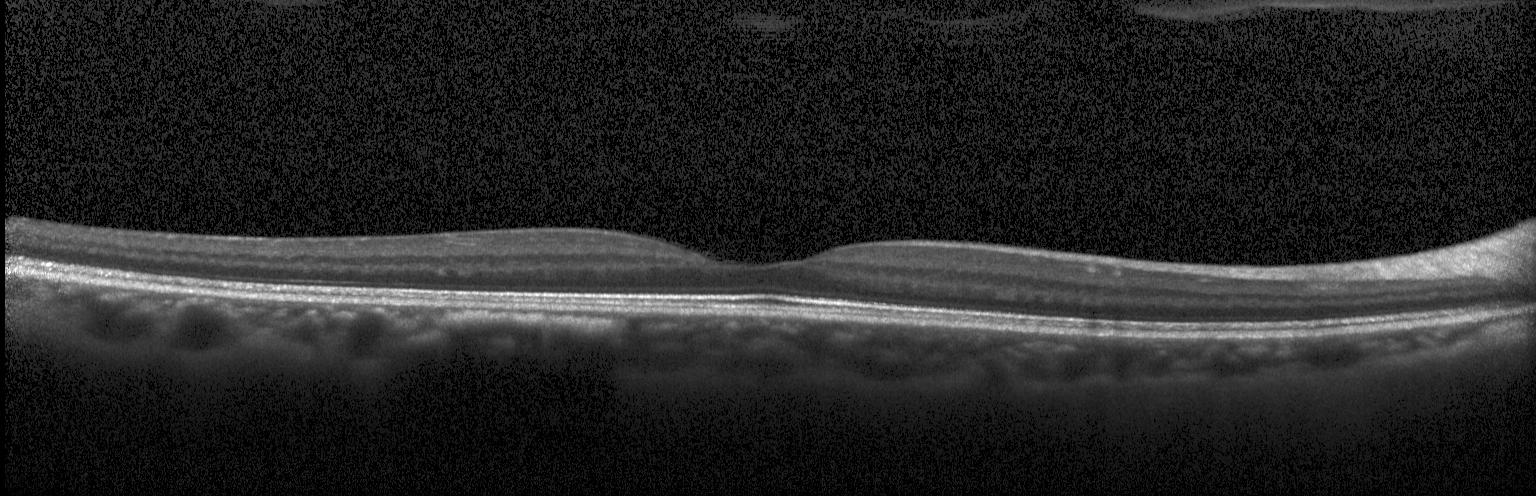
Retinal OCT cross-section
No choroidal neovascularization, diabetic macular edema, or drusen.